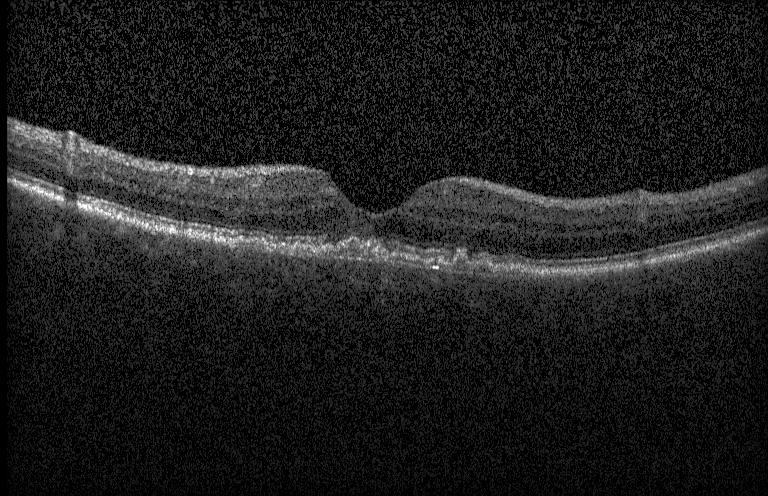
Impression: a choroidal neovascular membrane.